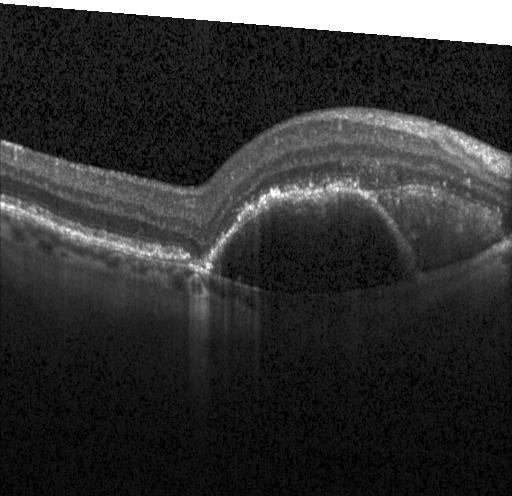
Retinal OCT cross-section showing choroidal neovascularization (CNV).